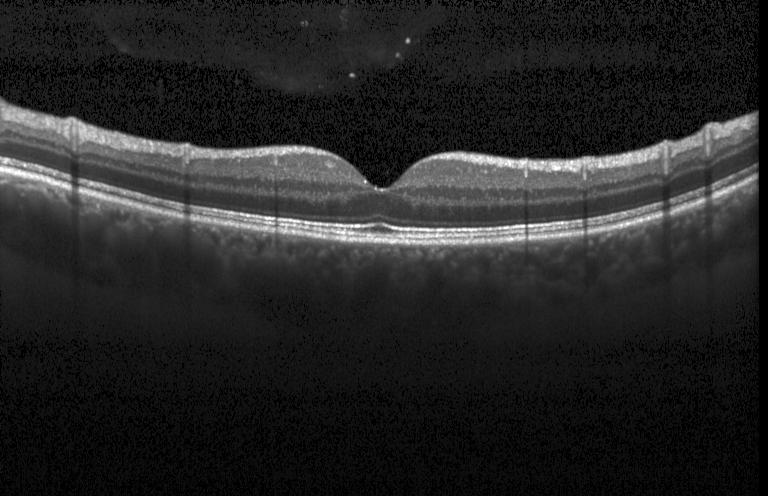 Instrument: Heidelberg Spectralis. Spectral-domain OCT. Retinal OCT cross-section. Through the macula.
This B-scan demonstrates no choroidal neovascularization, no diabetic macular edema, and no drusen.